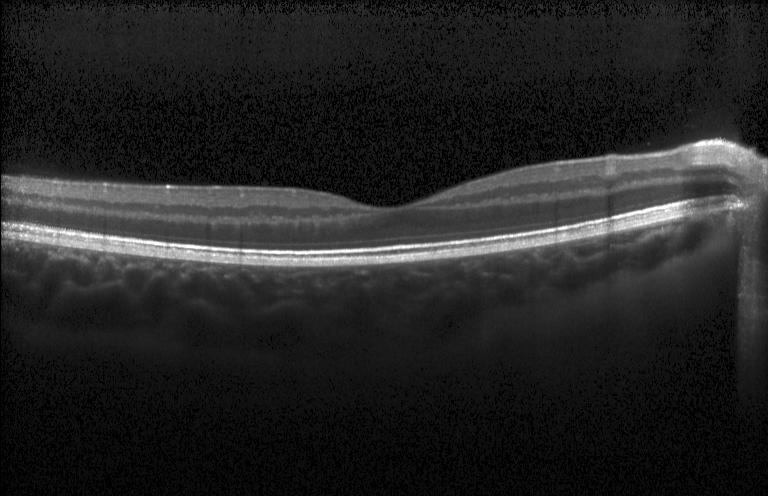 Optical coherence tomography scan; Heidelberg Spectralis OCT system; SD-OCT
Finding: no CNV, no DME, and no drusen.